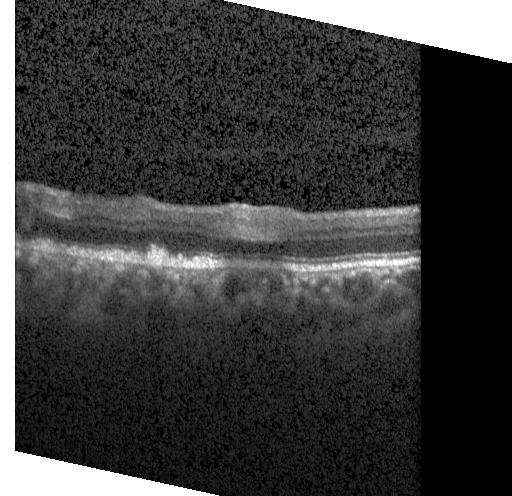 OCT line scan, fovea-centered, instrument: Heidelberg Spectralis. Diagnosis: drusen.